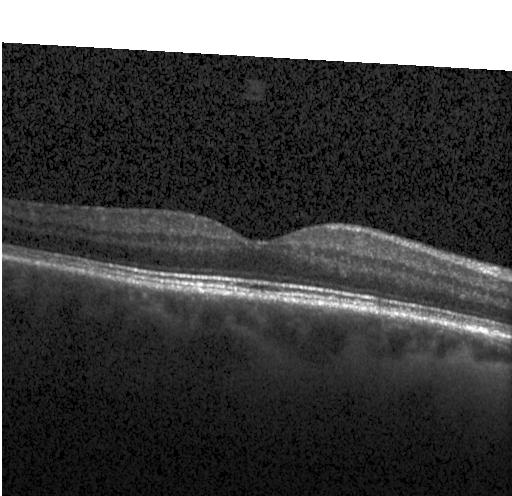 OCT finding: no evidence of choroidal neovascularization, diabetic macular edema, or drusen.